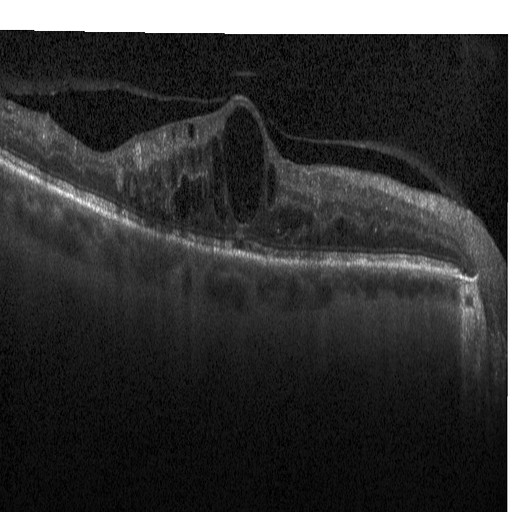
Retinal OCT cross-section; fovea-centered; Heidelberg Spectralis OCT system.
Diabetic macular edema (DME).